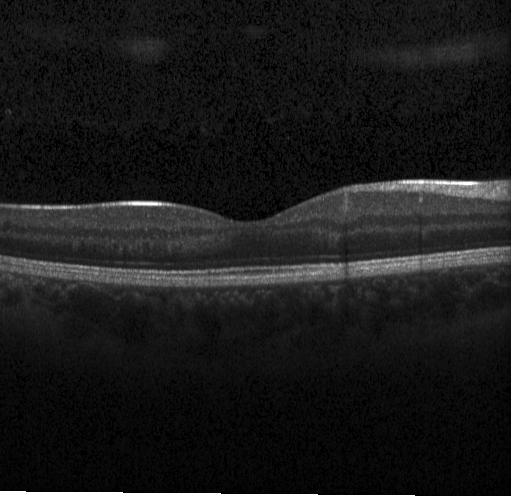
Spectral-domain optical coherence tomography, OCT line scan, centered on the fovea. No choroidal neovascularization, diabetic macular edema, or drusen.